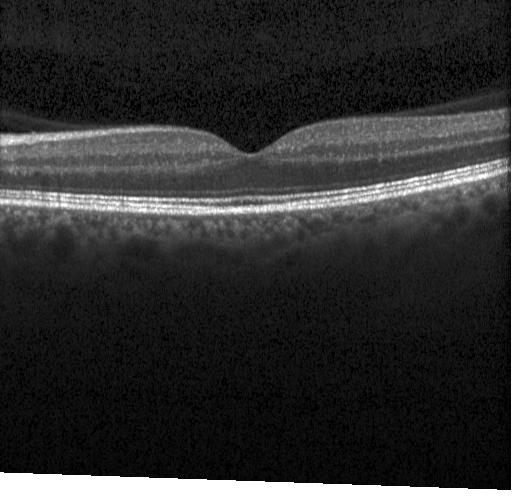 Through the macula · retinal OCT cross-section · spectral-domain OCT. Impression: no evidence of choroidal neovascularization, diabetic macular edema, or drusen.